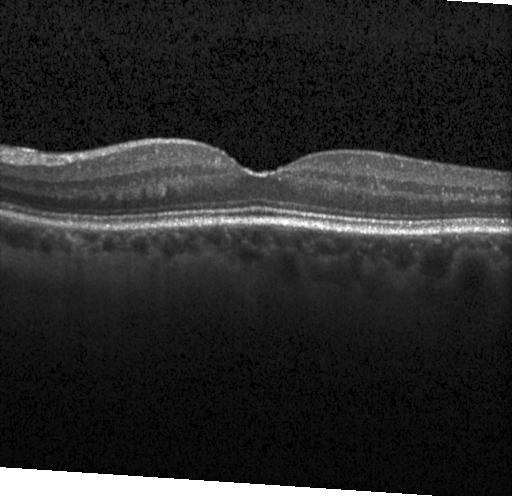

SD-OCT; through the macula; optical coherence tomography scan; acquired on a Heidelberg Spectralis. Assessment: neither CNV, DME, nor drusen.